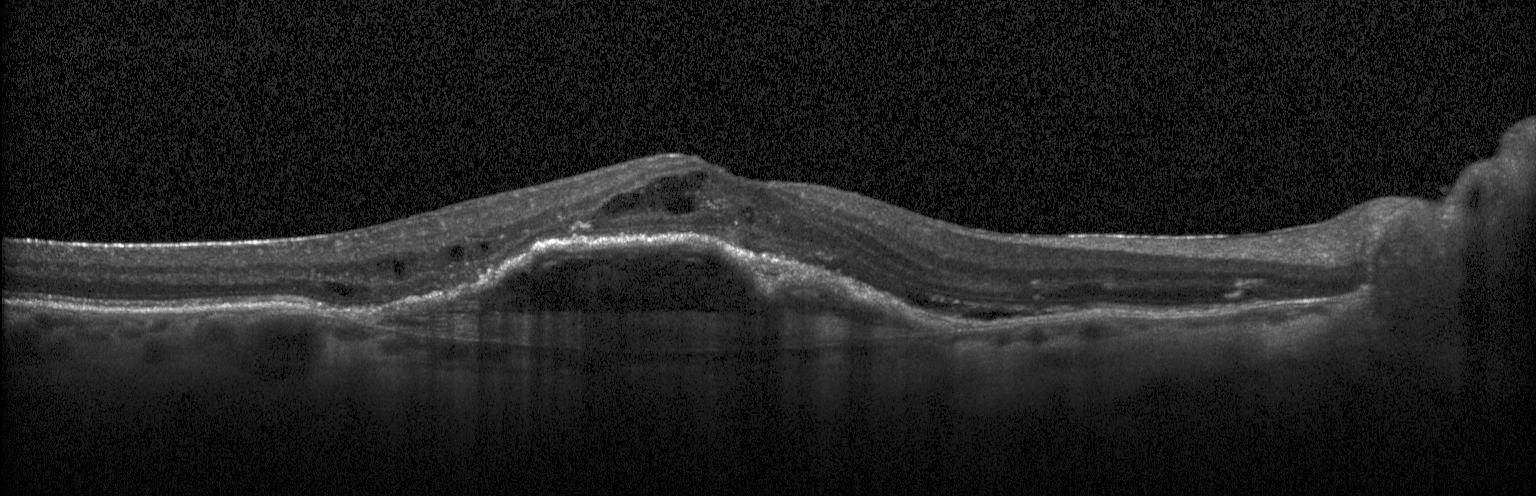
Acquired on a Heidelberg Spectralis; SD-OCT; OCT line scan
Finding: choroidal neovascularization.